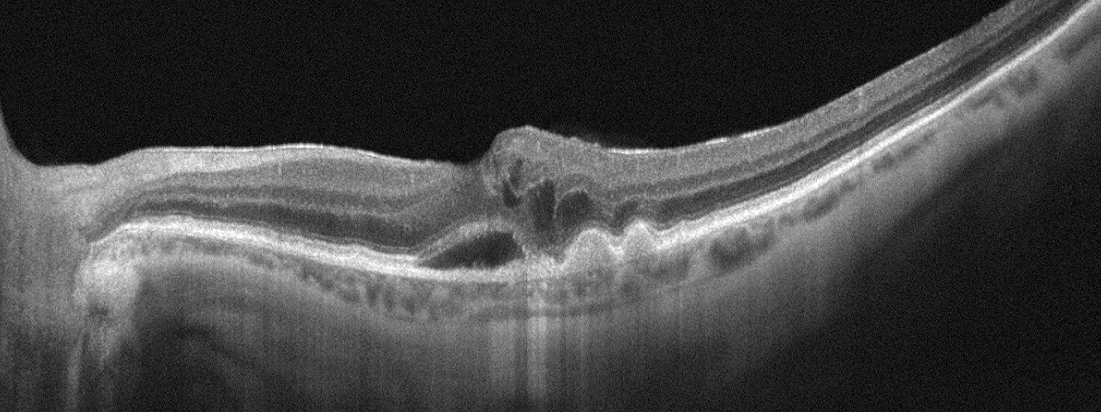
Diagnosis: age-related macular degeneration.